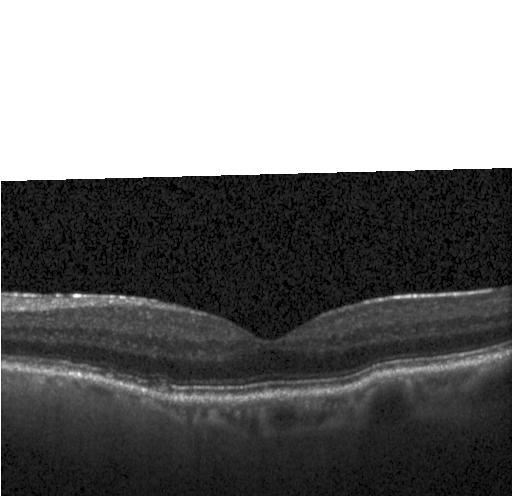
OCT line scan. OCT finding: multiple drusen.